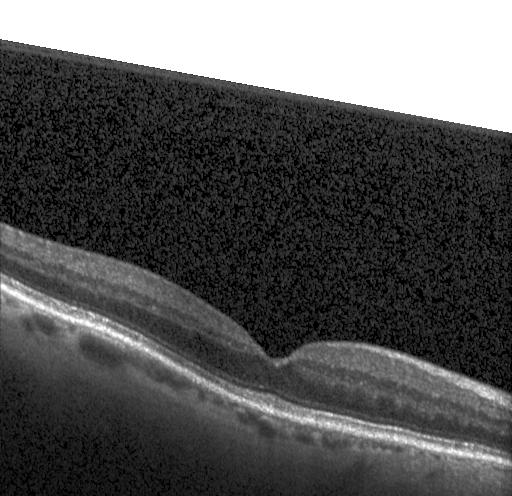

This B-scan demonstrates no evidence of choroidal neovascularization, diabetic macular edema, or drusen.